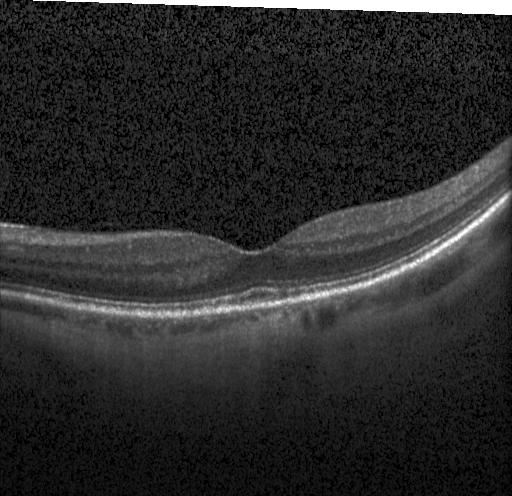

Optical coherence tomography B-scan — Impression: neither choroidal neovascularization, diabetic macular edema, nor drusen.